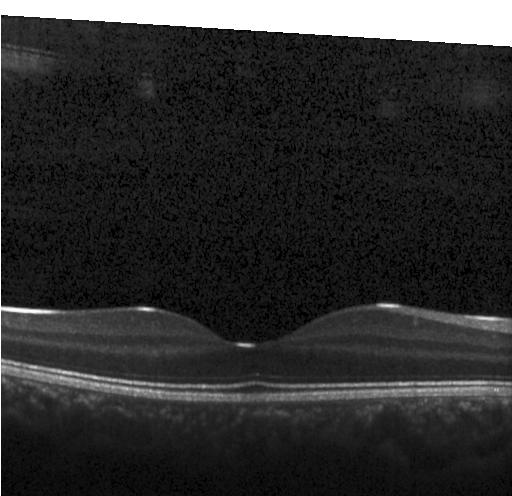 Spectral-domain OCT, fovea-centered, OCT B-scan. Finding: neither choroidal neovascularization, diabetic macular edema, nor drusen.